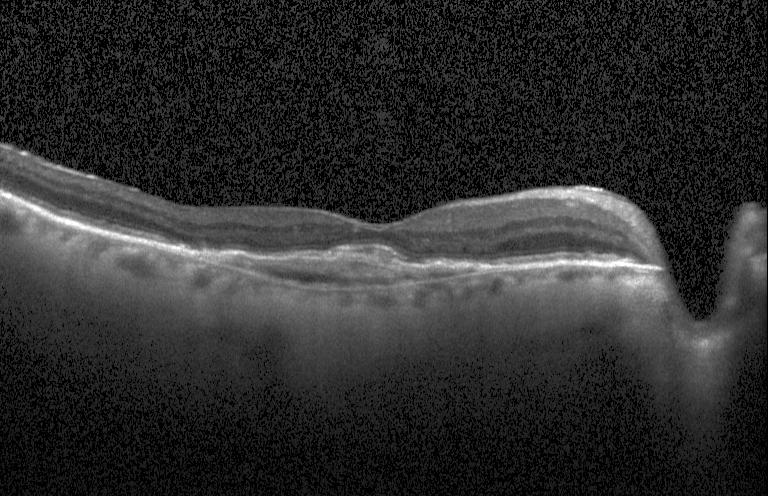
Optical coherence tomography scan, macular scan
OCT finding: CNV.